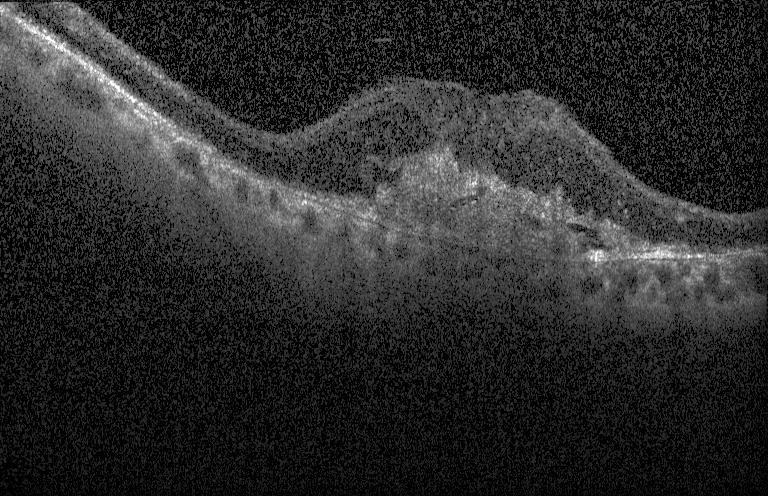

Centered on the fovea. OCT B-scan. Acquired on a Heidelberg Spectralis.
Finding: a choroidal neovascular membrane.